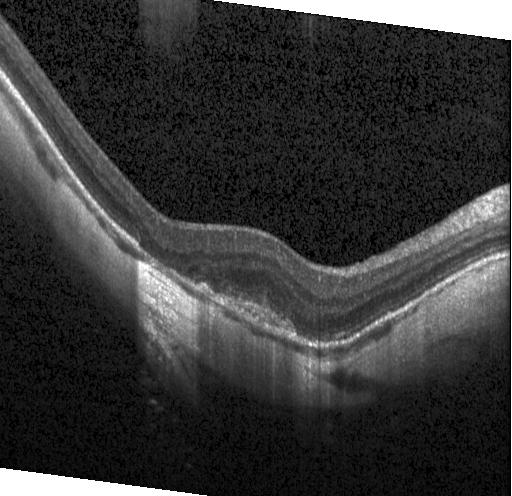 OCT line scan. Centered on the fovea. Heidelberg Spectralis OCT system — This B-scan demonstrates a choroidal neovascular membrane.